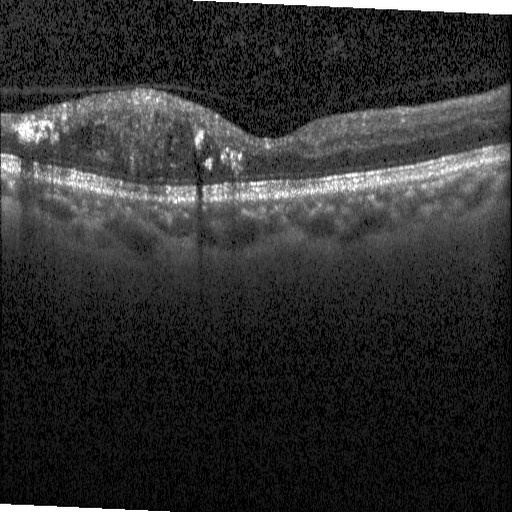

Optical coherence tomography scan — The scan shows diabetic macular edema.